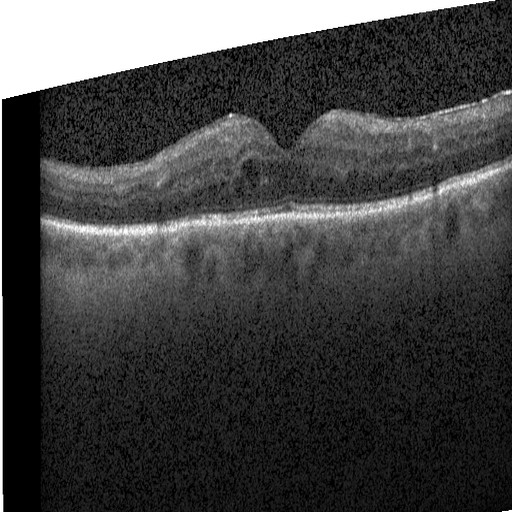

Finding: diabetic macular edema (DME).